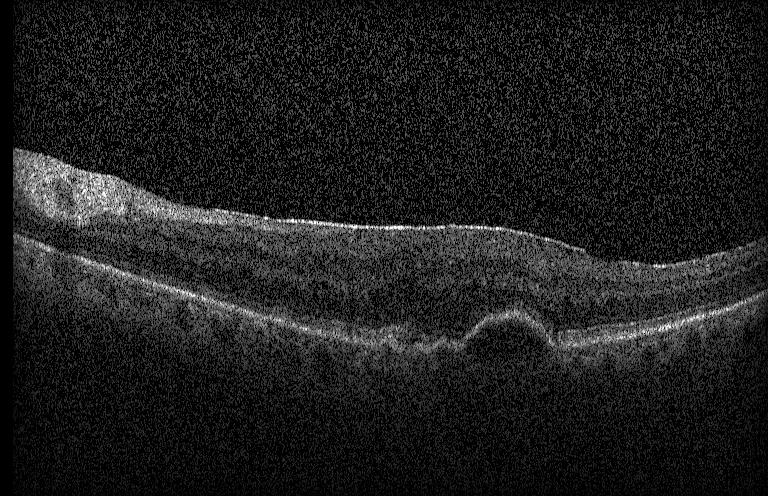 Spectral-domain optical coherence tomography, through the macula, instrument: Heidelberg Spectralis, OCT line scan.
Diagnosis: a choroidal neovascular membrane.